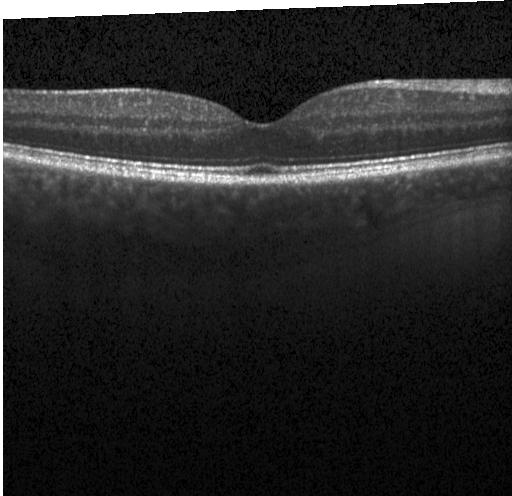

Fovea-centered. Retinal OCT cross-section. Spectral-domain optical coherence tomography — Finding: neither choroidal neovascularization, diabetic macular edema, nor drusen.